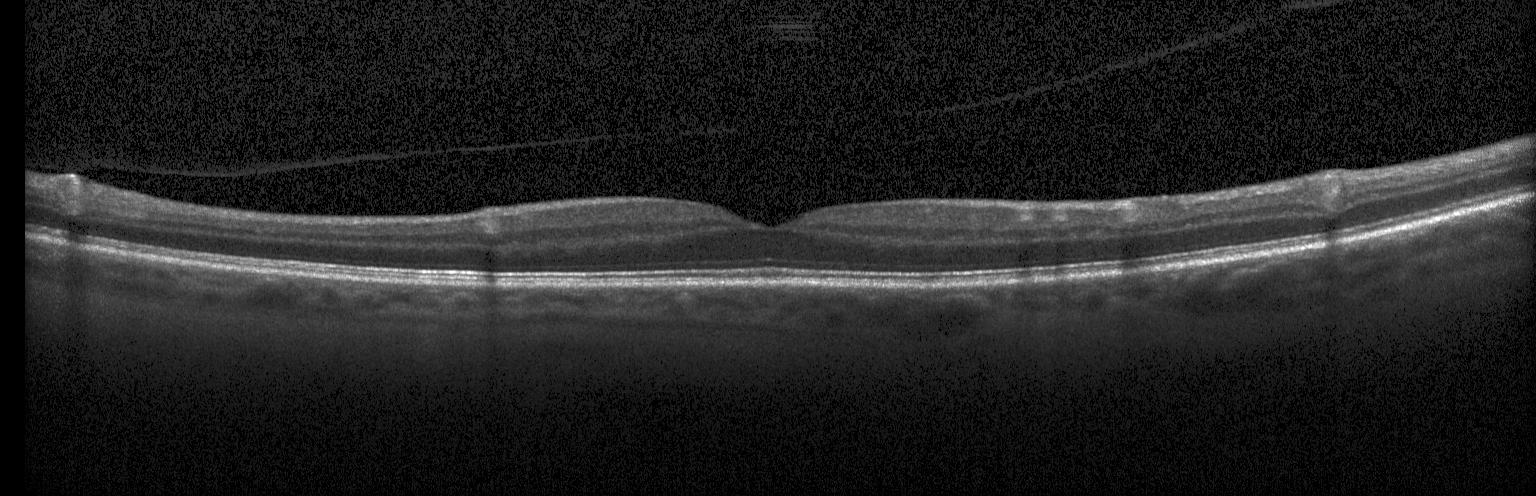
Spectral-domain OCT B-scan: neither CNV, DME, nor drusen.